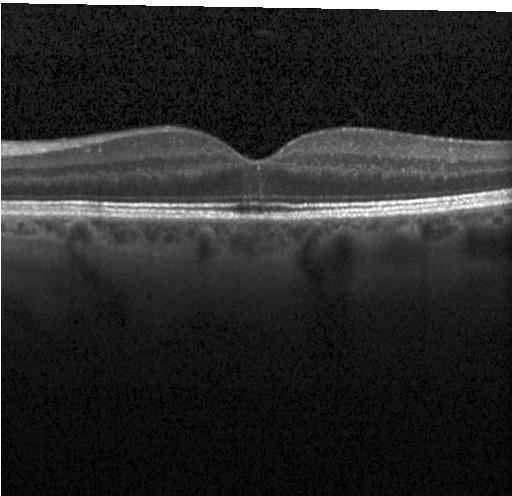
OCT line scan
This B-scan demonstrates no choroidal neovascularization, diabetic macular edema, or drusen.